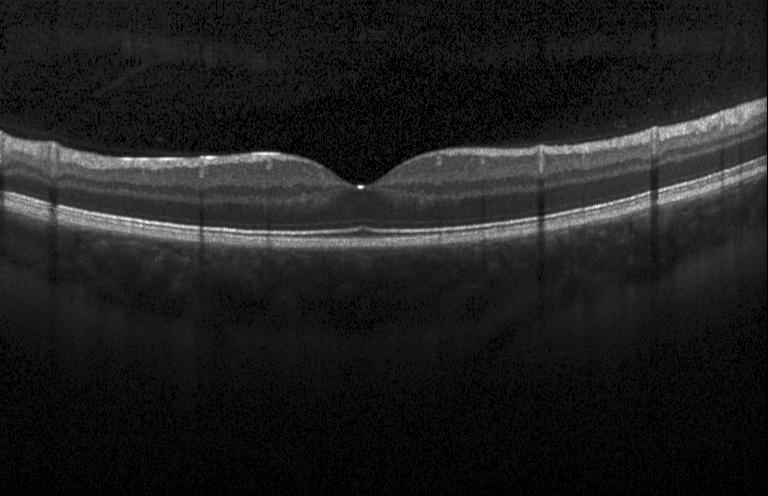 Retinal OCT cross-section
Macular OCT: no choroidal neovascularization, diabetic macular edema, or drusen.